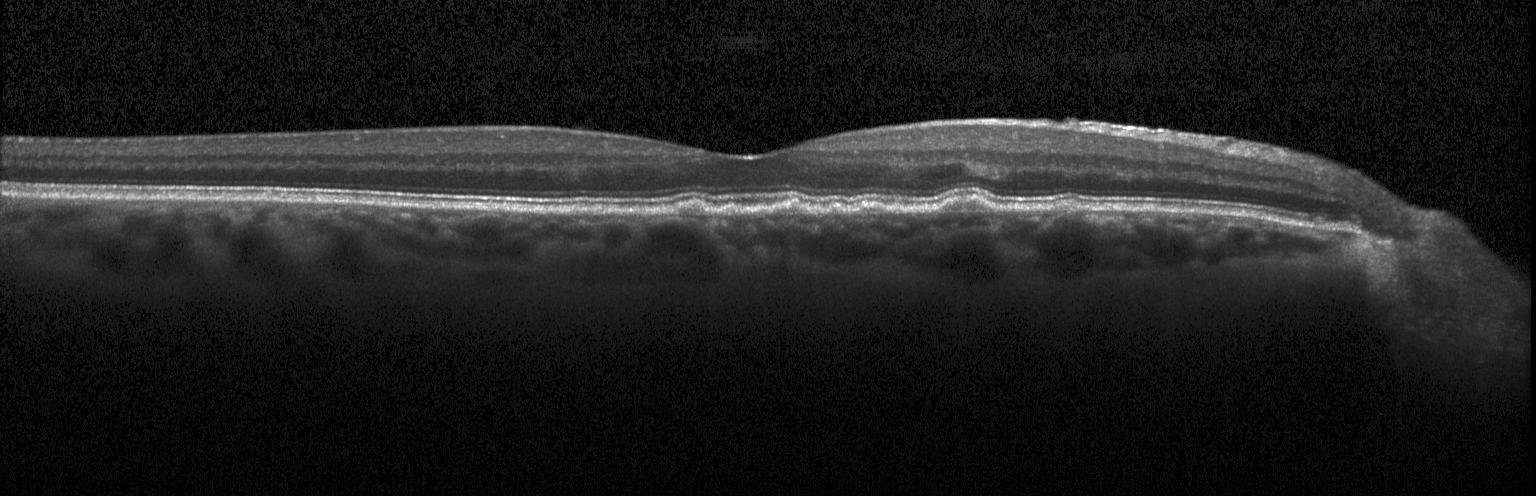

Fovea-centered, retinal OCT cross-section, instrument: Heidelberg Spectralis
This B-scan demonstrates multiple drusen.